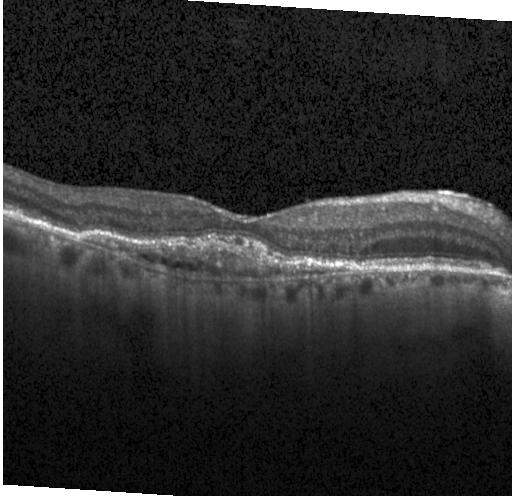

OCT line scan; Heidelberg Spectralis OCT system; through the macula. Dx: choroidal neovascularization.